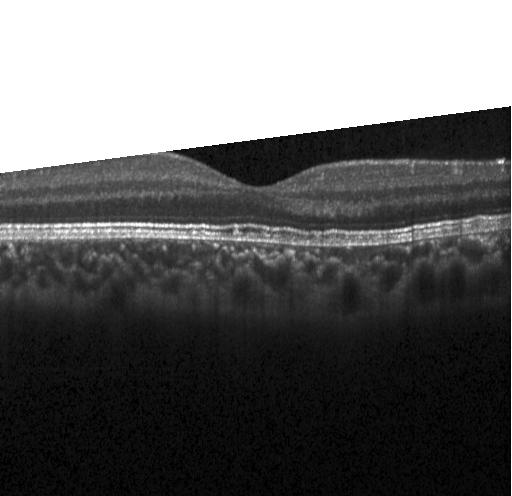

Impression: neither CNV, DME, nor drusen.